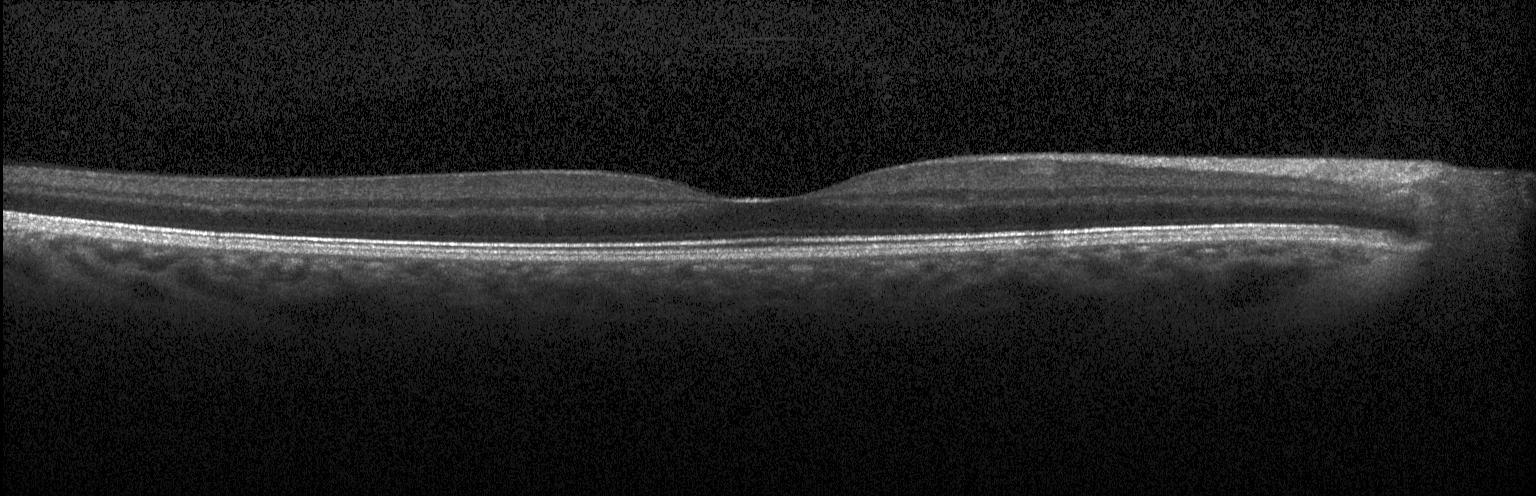

Diagnosis: no CNV, no DME, and no drusen.